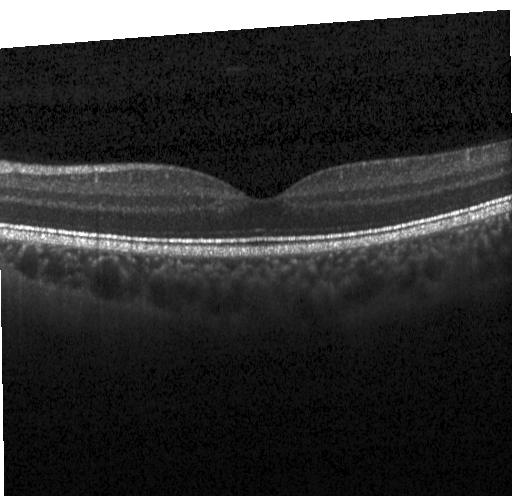 Fovea-centered · optical coherence tomography scan — Finding: no choroidal neovascularization, diabetic macular edema, or drusen.